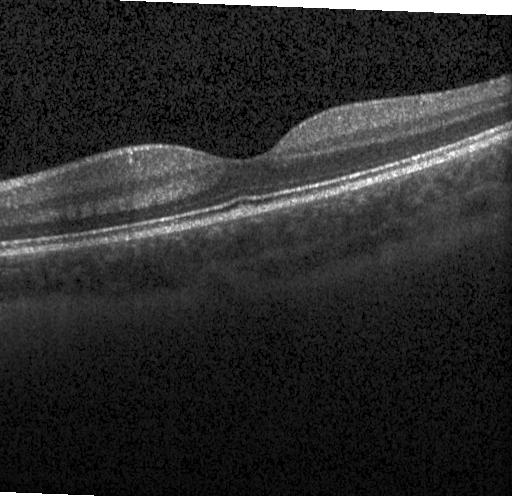
Diagnosis: neither CNV, DME, nor drusen.